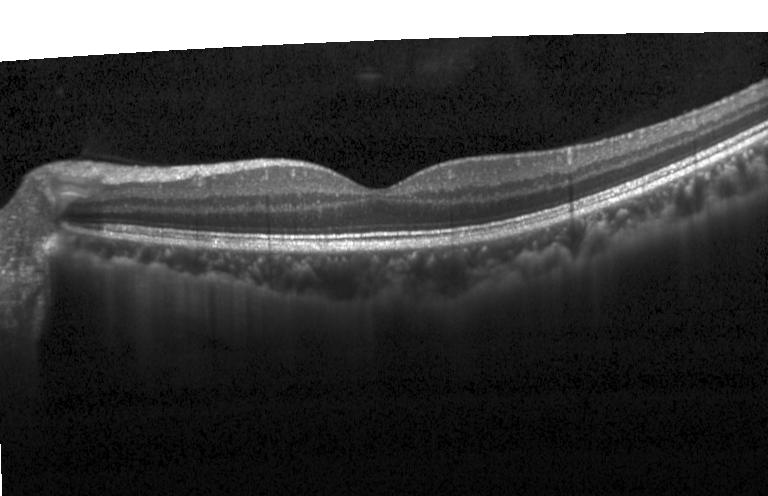

Impression: no choroidal neovascularization, diabetic macular edema, or drusen.